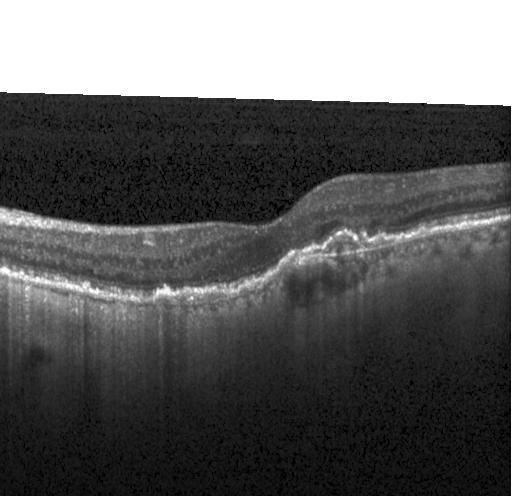
Optical coherence tomography scan. Instrument: Heidelberg Spectralis. Centered on the fovea. SD-OCT.
Finding: a choroidal neovascular membrane.